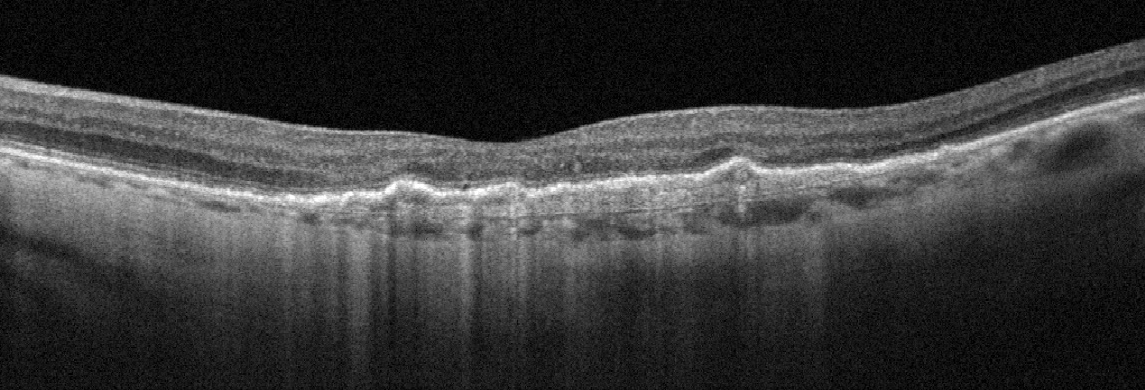
OCT B-scan, instrument: Optovue Avanti RTVue XR, macular scan — Assessment: age-related macular degeneration (AMD).